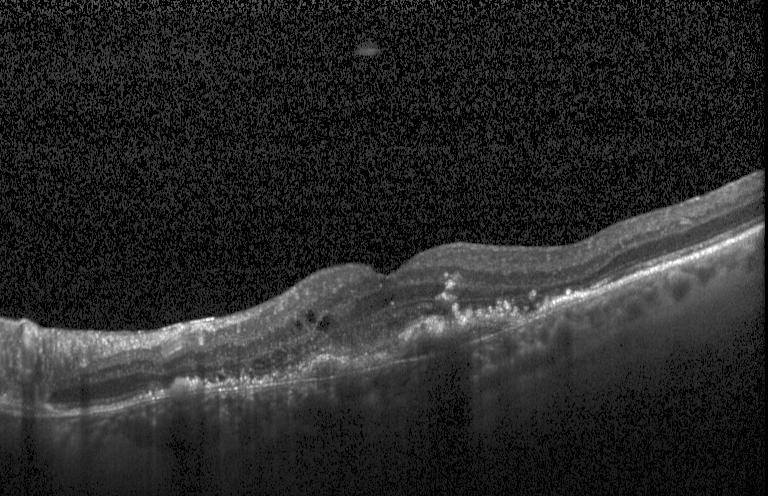
This B-scan demonstrates a choroidal neovascular membrane.